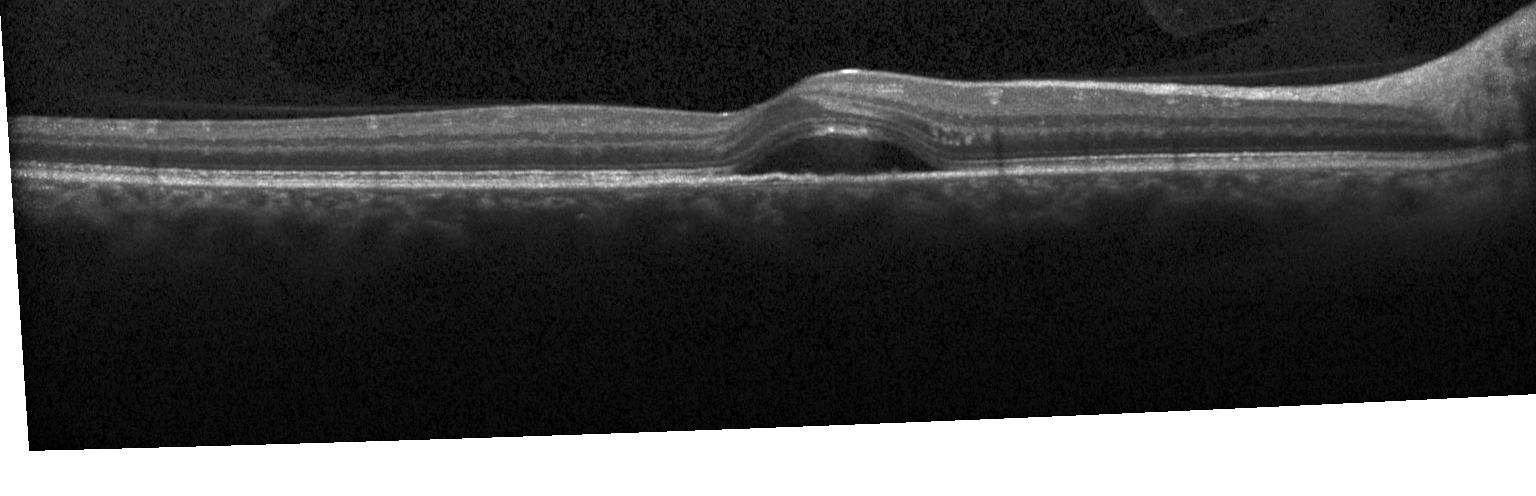

OCT B-scan, spectral-domain OCT, Heidelberg Spectralis OCT system. Finding: CNV.